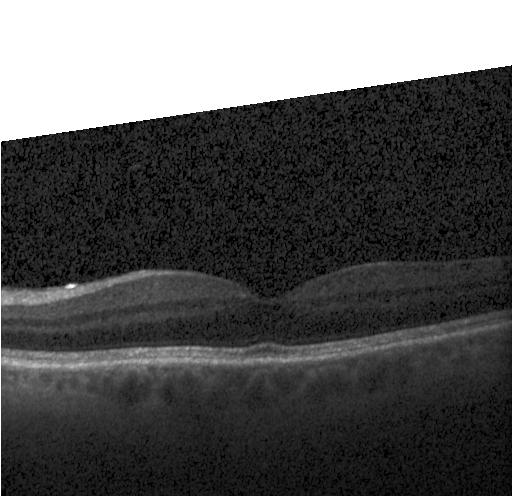 SD-OCT; retinal OCT B-scan — Dx: no evidence of choroidal neovascularization, diabetic macular edema, or drusen.